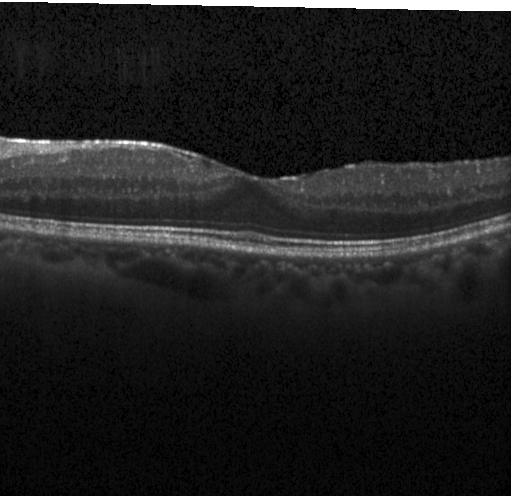 Horizontal scan through the fovea, OCT B-scan, spectral-domain OCT. OCT finding: neither CNV, DME, nor drusen.